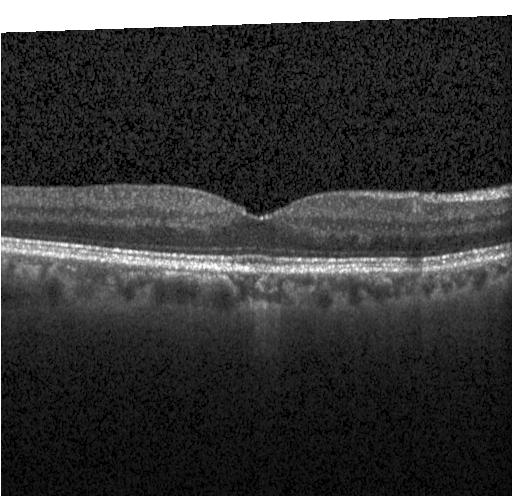
Dx: no evidence of CNV, DME, or drusen.